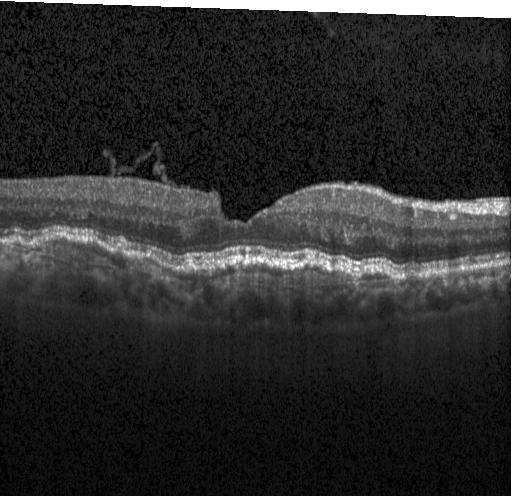
Finding: choroidal neovascularization (CNV).